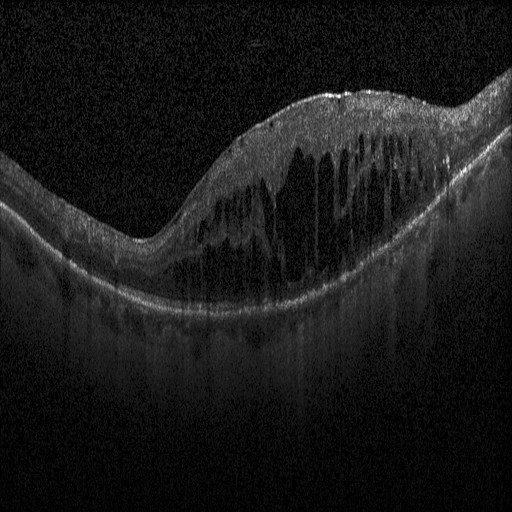 OCT B-scan showing DME.